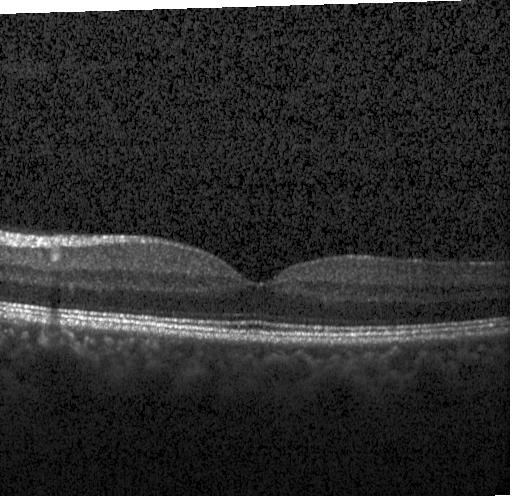
Fovea-centered · OCT B-scan. Finding: no evidence of CNV, DME, or drusen.